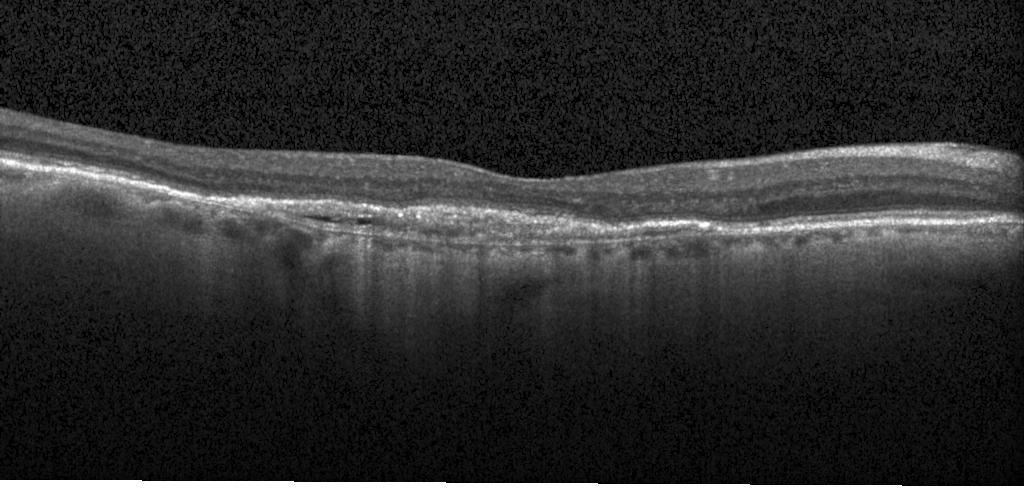

Finding: choroidal neovascularization.